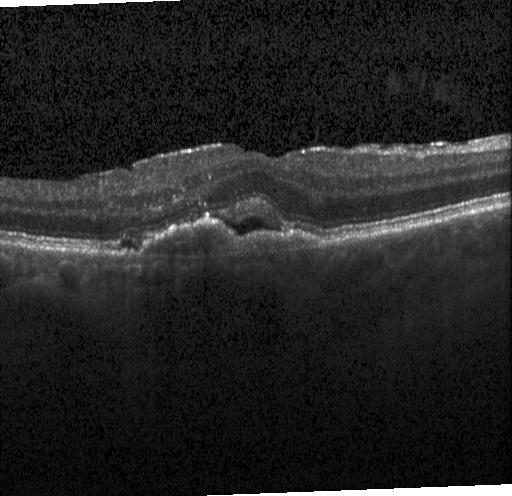

Finding: a choroidal neovascular membrane.